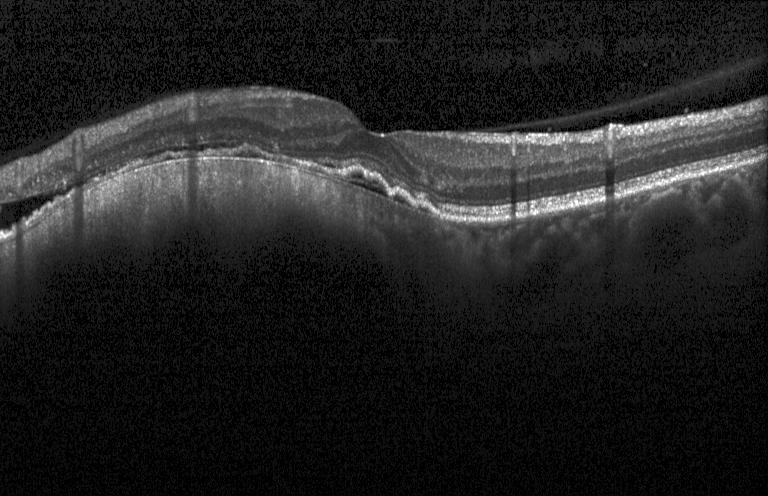

OCT B-scan showing choroidal neovascularization (CNV).